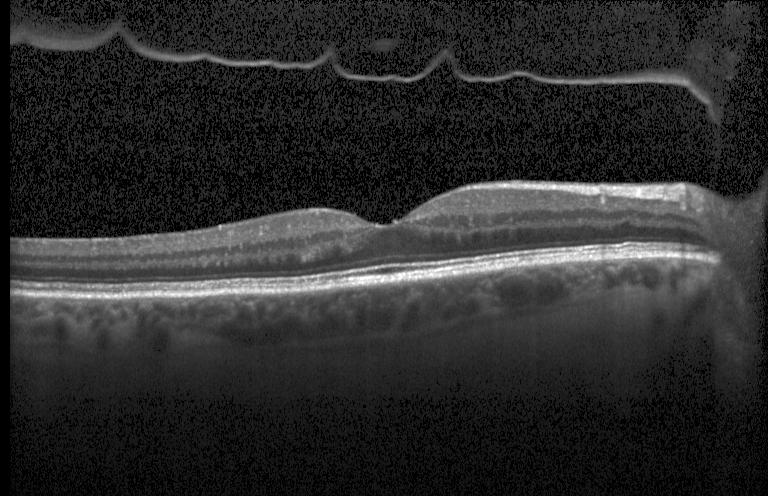
OCT B-scan — Finding: neither choroidal neovascularization, diabetic macular edema, nor drusen.